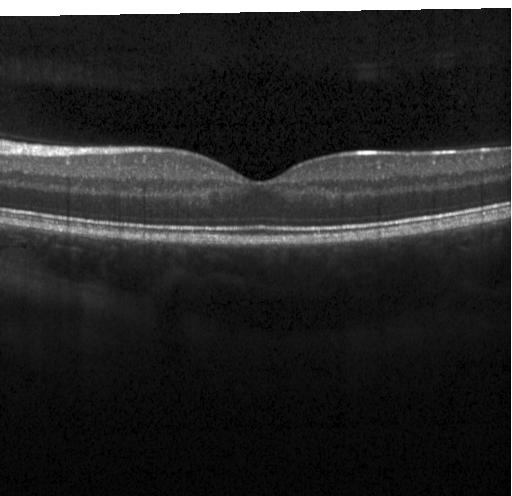
No choroidal neovascularization, no diabetic macular edema, and no drusen.